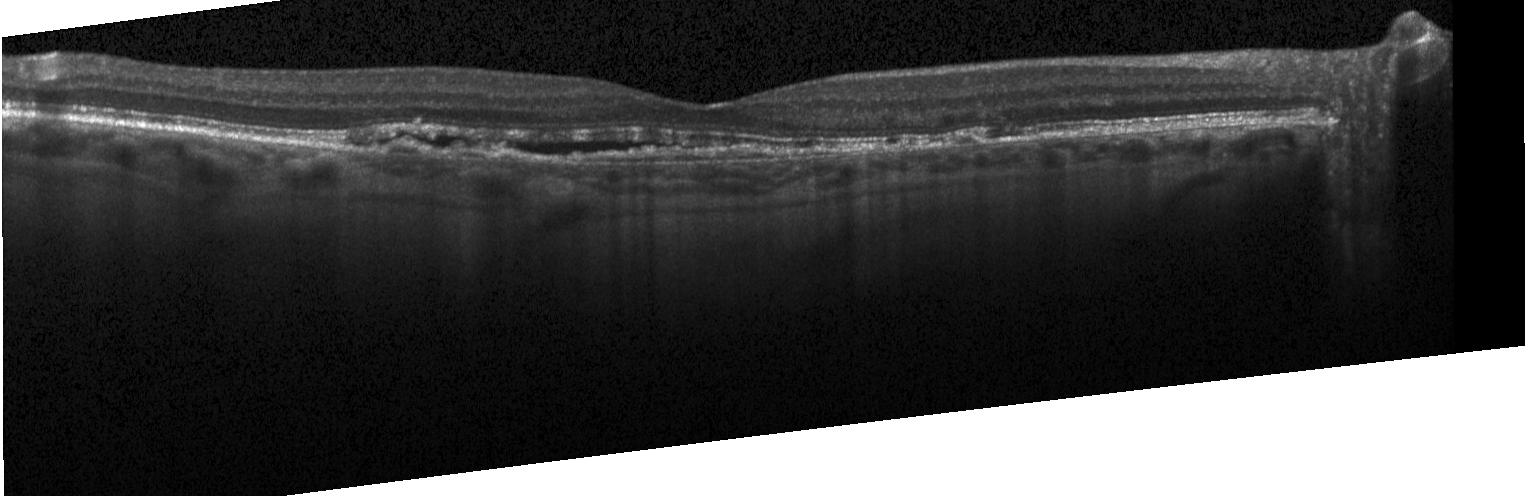
Retinal OCT B-scan, macular scan.
Diagnosis: choroidal neovascularization.